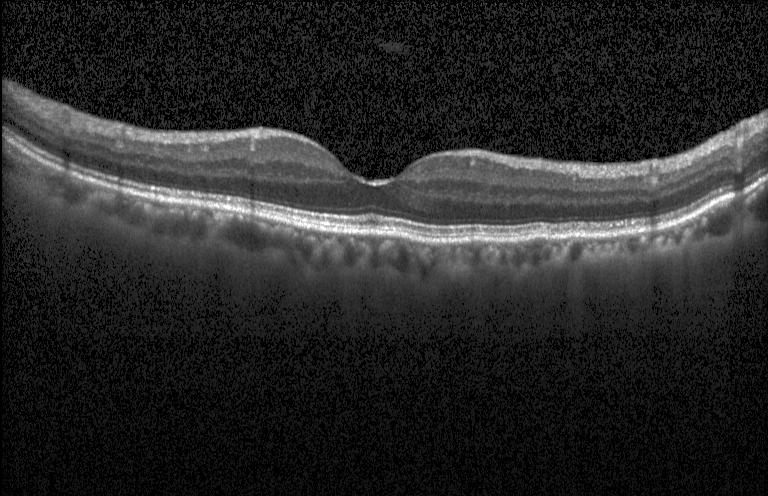 SD-OCT, centered on the fovea, retinal OCT B-scan, acquired on a Heidelberg Spectralis
Macular OCT: no CNV, DME, or drusen.